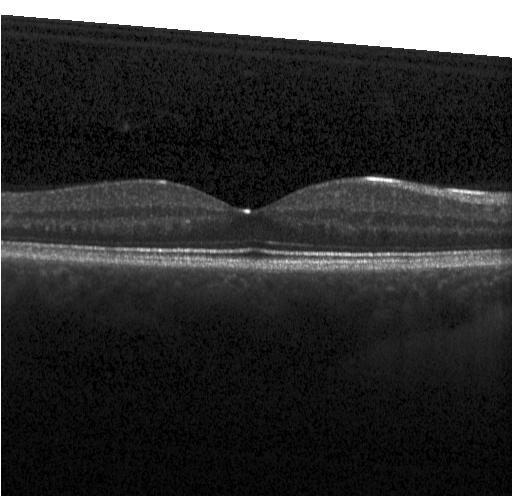
Macular scan, optical coherence tomography scan, spectral-domain OCT — No CNV, no DME, and no drusen.